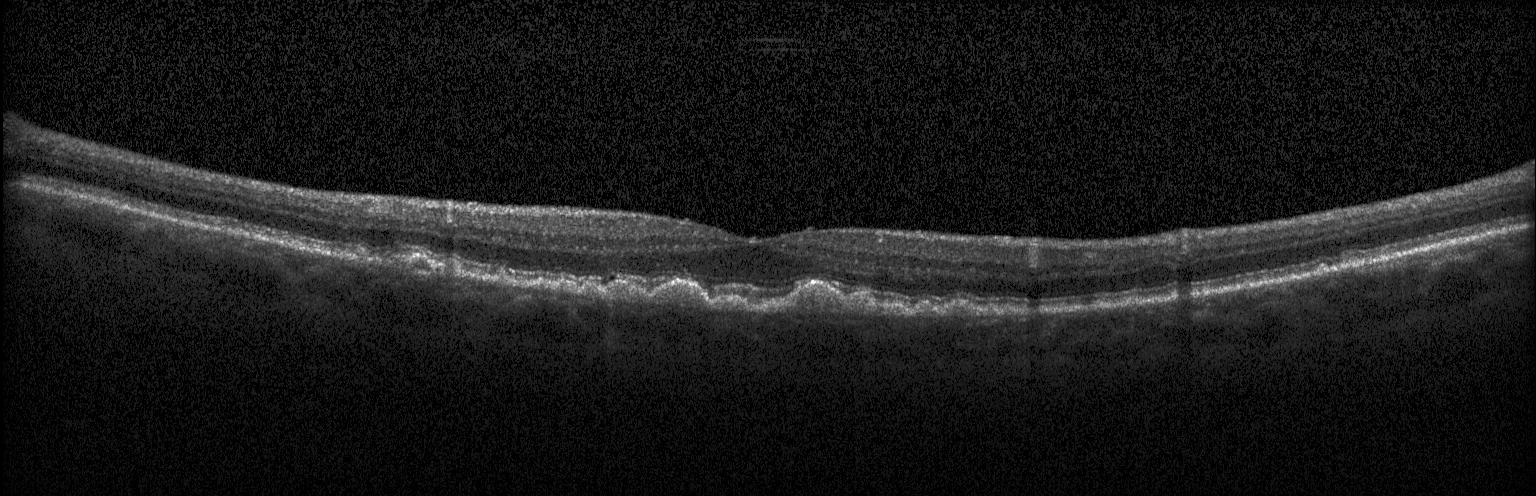

Heidelberg Spectralis OCT system · spectral-domain OCT · optical coherence tomography scan. Finding: drusen.